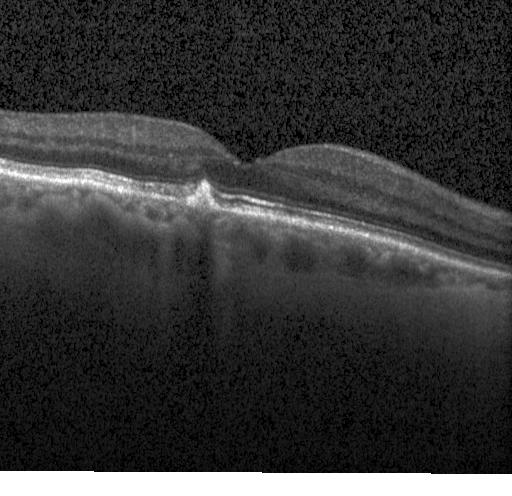 Optical coherence tomography scan; Heidelberg Spectralis OCT system; fovea-centered; SD-OCT
Finding: multiple drusen.